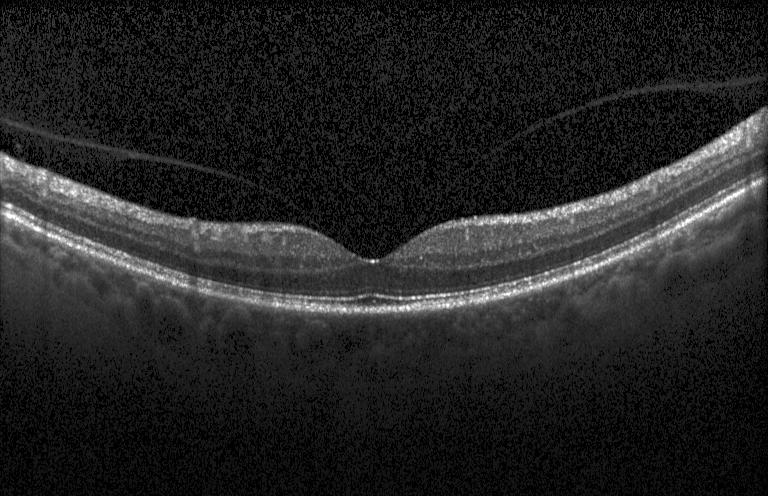 OCT line scan. Acquired on a Heidelberg Spectralis — The scan shows no choroidal neovascularization, diabetic macular edema, or drusen.